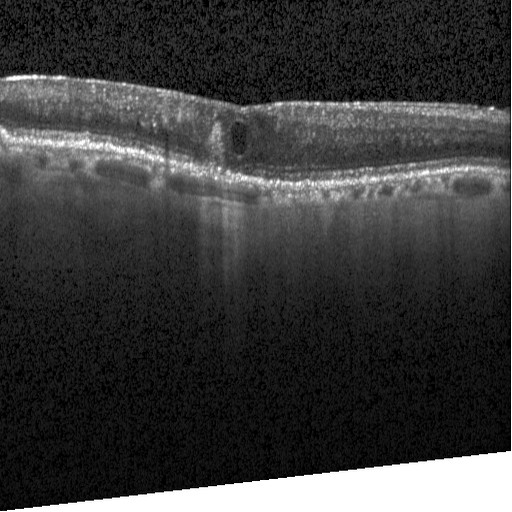 Through the macula, spectral-domain OCT, retinal OCT B-scan, instrument: Heidelberg Spectralis.
Dx: DME.